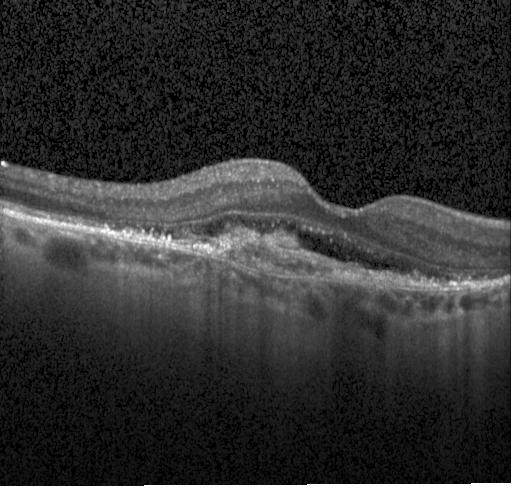
OCT line scan
Diagnosis: choroidal neovascularization (CNV).